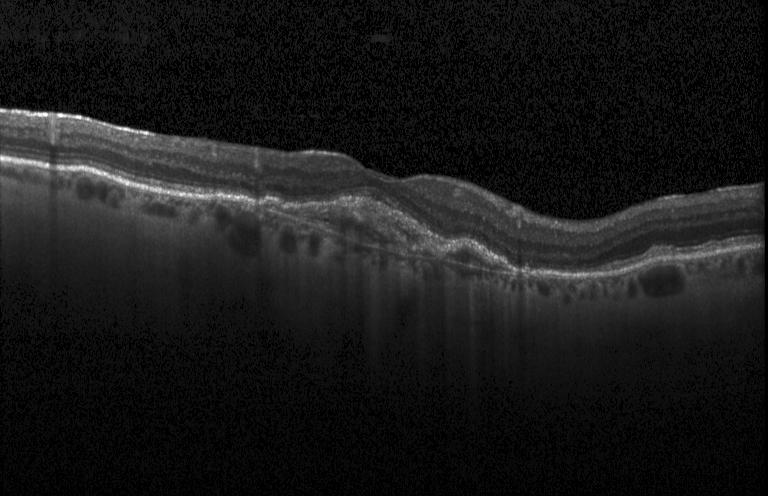 Spectral-domain optical coherence tomography. OCT B-scan — This B-scan demonstrates a choroidal neovascular membrane.